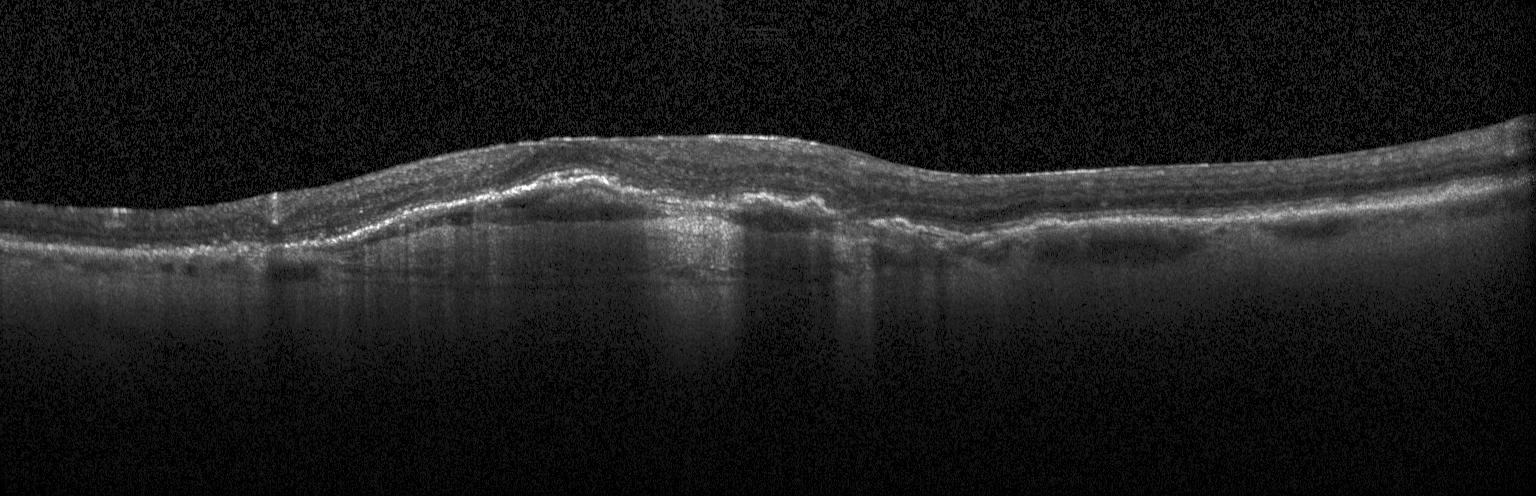 Macular scan; SD-OCT; instrument: Heidelberg Spectralis; optical coherence tomography B-scan — Dx: CNV.